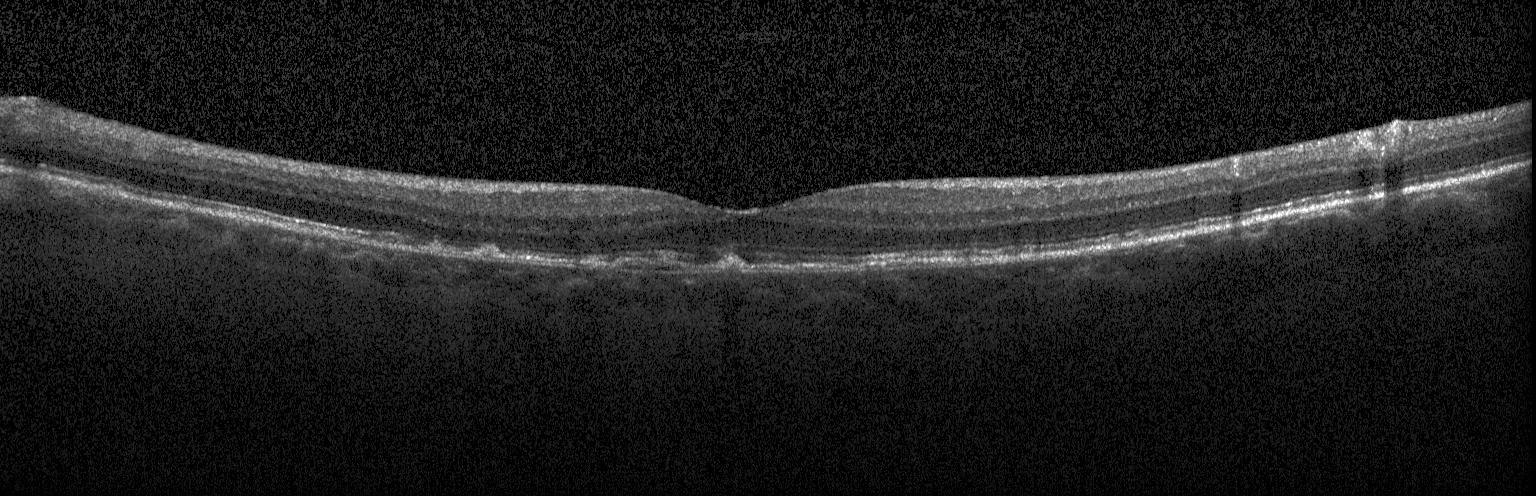 Through the macula; OCT B-scan — Dx: a choroidal neovascular membrane.